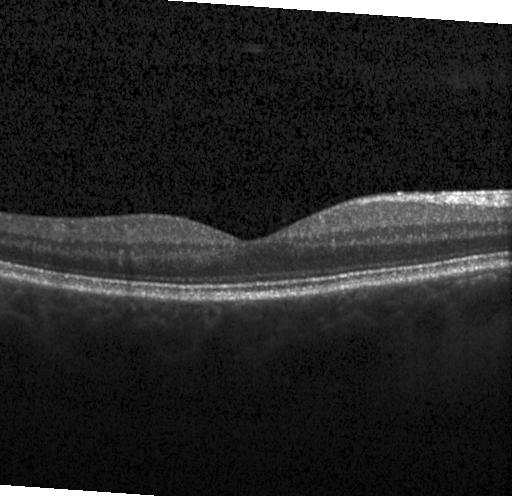

OCT scan showing neither choroidal neovascularization, diabetic macular edema, nor drusen.